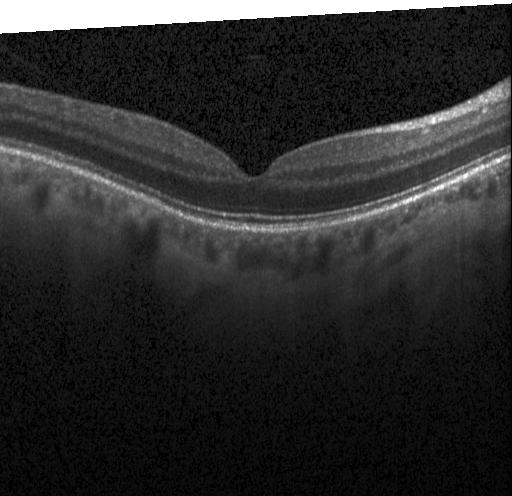
OCT finding: no CNV, no DME, and no drusen.